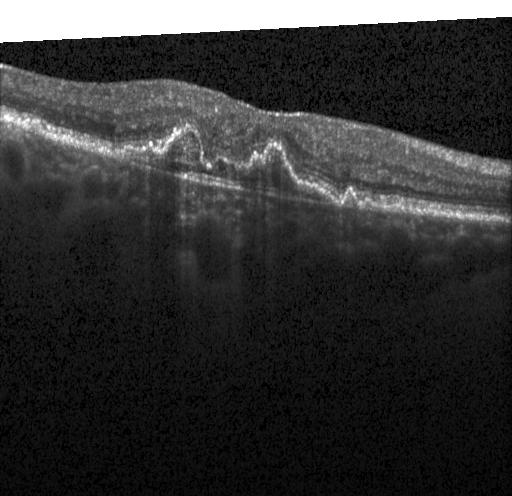 OCT finding: CNV.